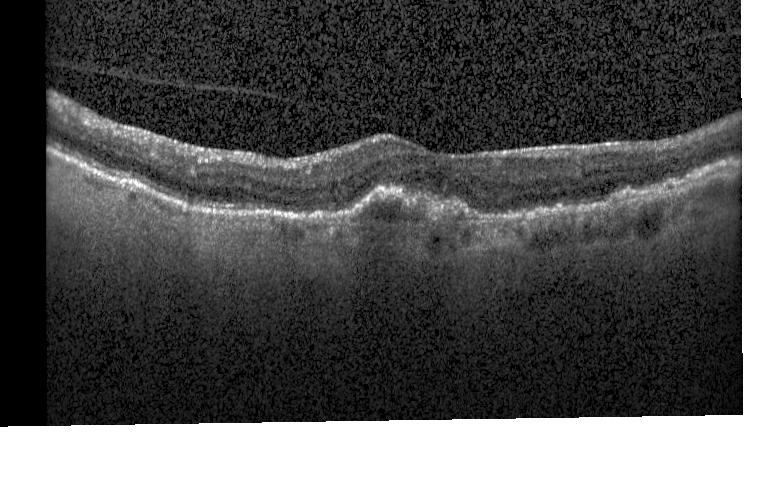

Assessment: choroidal neovascularization (CNV).